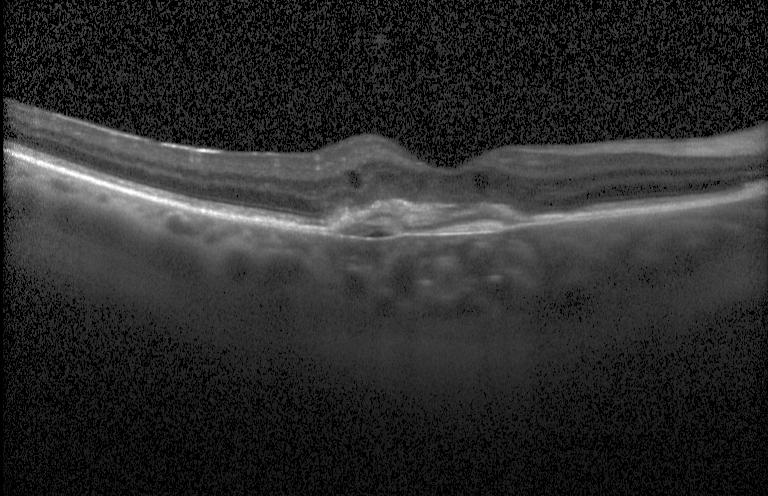

SD-OCT. Acquired on a Heidelberg Spectralis. Optical coherence tomography scan. Fovea-centered — The scan shows choroidal neovascularization.